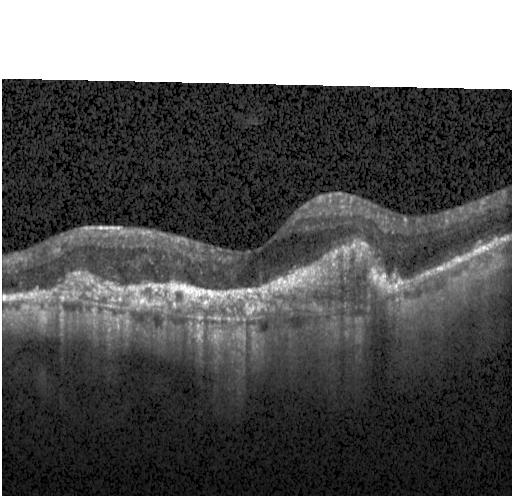
OCT B-scan. A choroidal neovascular membrane.